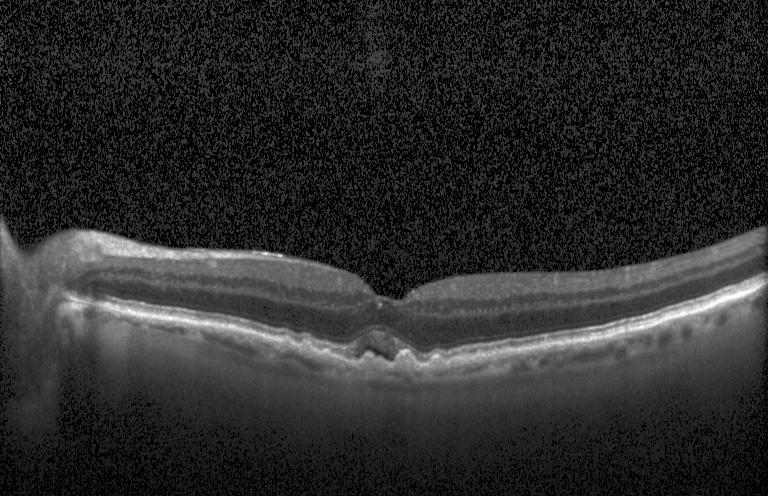
OCT finding: choroidal neovascularization (CNV).